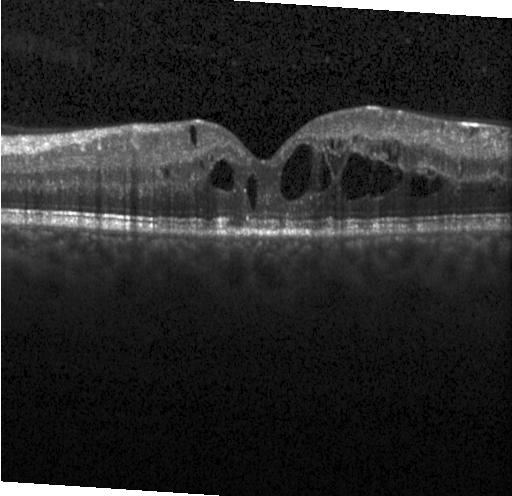 Dx: diabetic macular edema (DME).